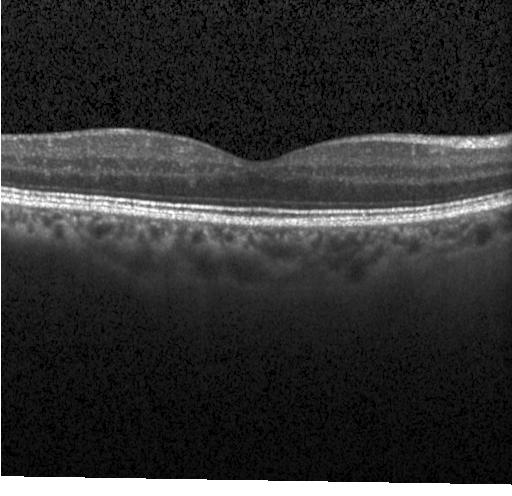
SD-OCT, OCT line scan. Diagnosis: no CNV, no DME, and no drusen.